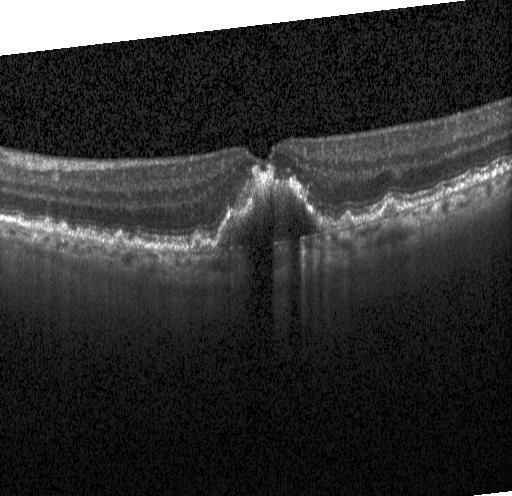

Spectral-domain OCT · optical coherence tomography scan — OCT finding: choroidal neovascularization (CNV).